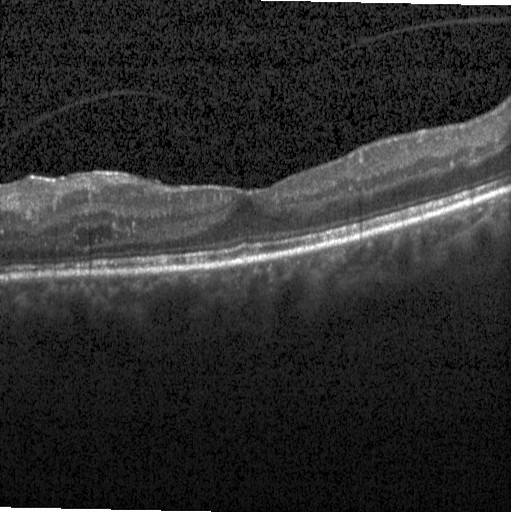 Acquired on a Heidelberg Spectralis, optical coherence tomography scan. Impression: DME.